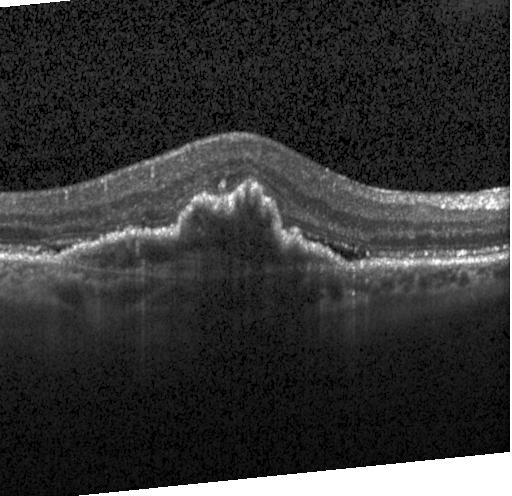 Optical coherence tomography scan. SD-OCT. Acquired on a Heidelberg Spectralis
Diagnosis: choroidal neovascularization (CNV).